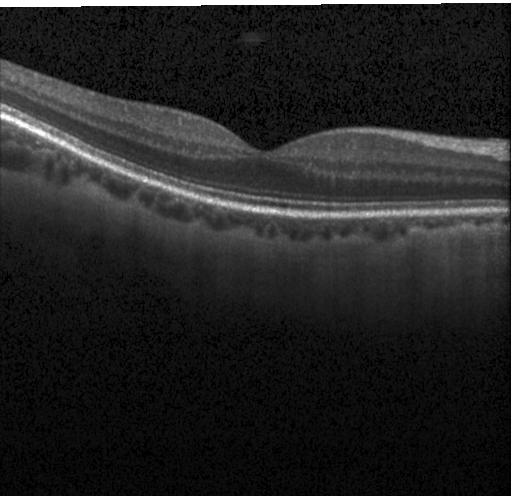 Optical coherence tomography B-scan, centered on the fovea, Heidelberg Spectralis OCT system
Impression: no evidence of CNV, DME, or drusen.